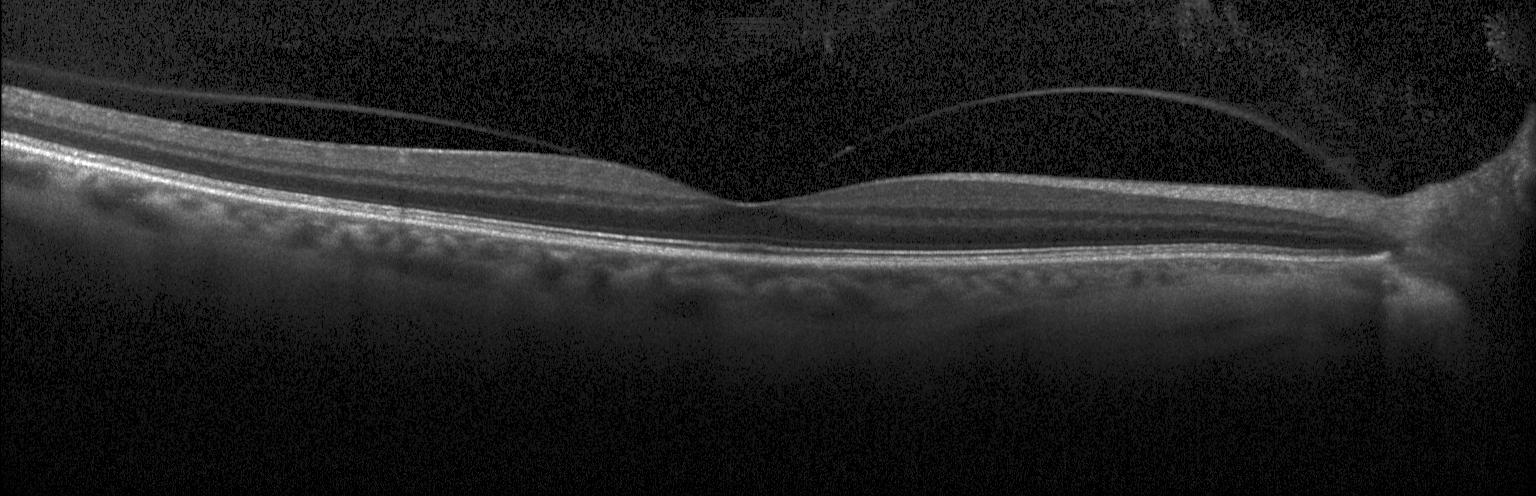 OCT line scan, spectral-domain optical coherence tomography, acquired on a Heidelberg Spectralis — This B-scan demonstrates no evidence of CNV, DME, or drusen.